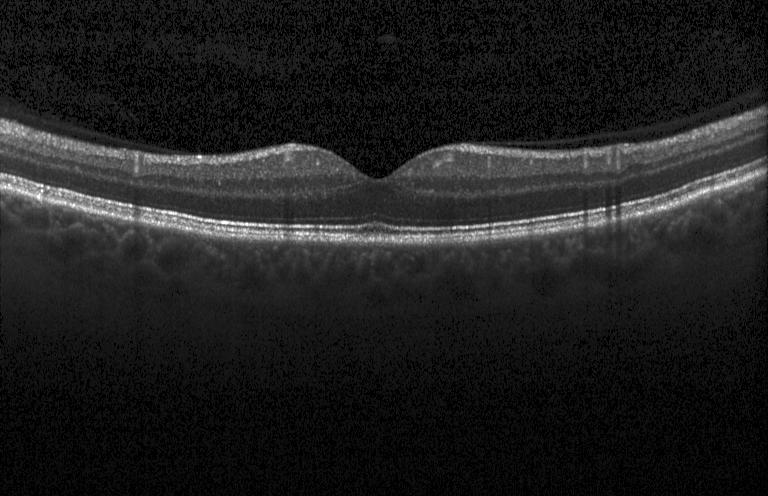
SD-OCT; retinal OCT B-scan. Impression: no evidence of choroidal neovascularization, diabetic macular edema, or drusen.